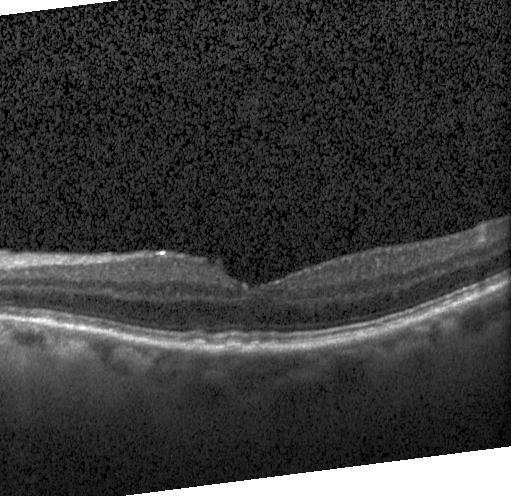 Macular OCT: drusen.